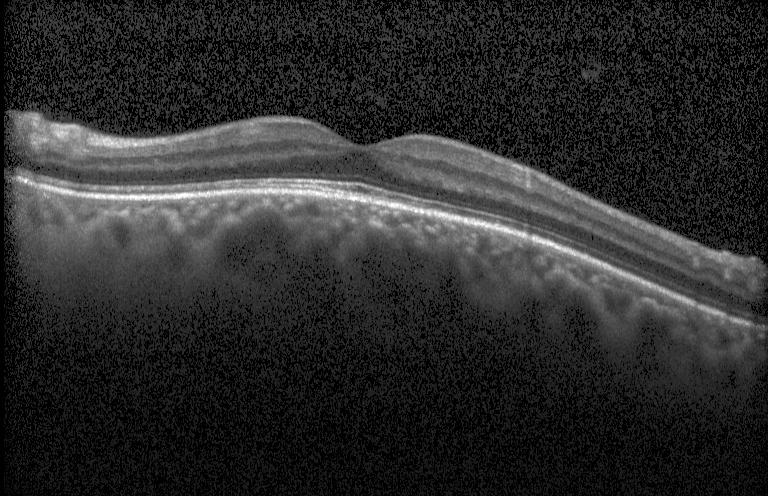

Centered on the fovea; Heidelberg Spectralis OCT system; spectral-domain optical coherence tomography; retinal OCT cross-section — Finding: no choroidal neovascularization, diabetic macular edema, or drusen.